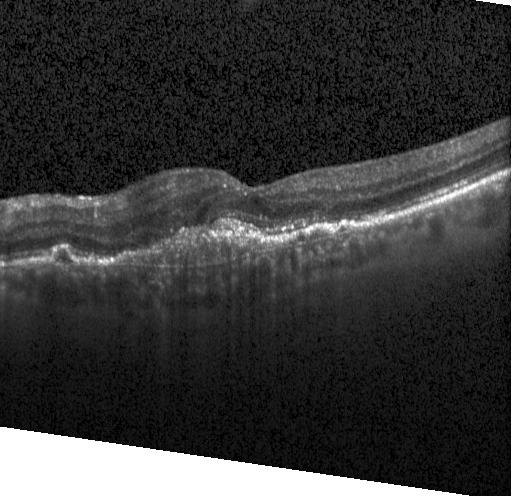
Impression: a choroidal neovascular membrane.